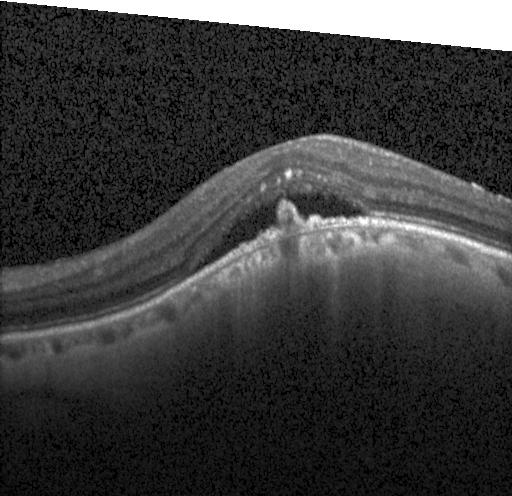
Retinal OCT B-scan, macular scan, SD-OCT, Heidelberg Spectralis OCT system
OCT finding: a choroidal neovascular membrane.